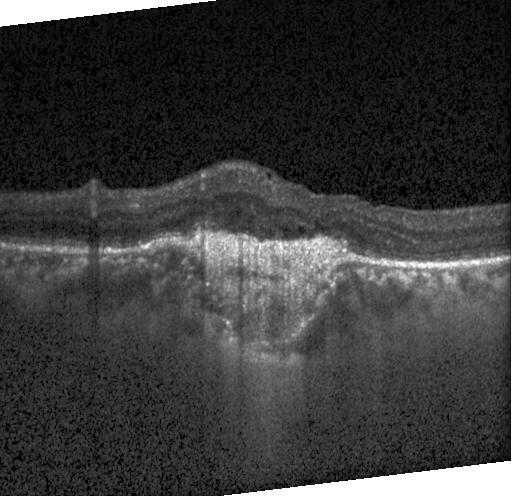

Optical coherence tomography B-scan · spectral-domain OCT · Heidelberg Spectralis
Impression: CNV.